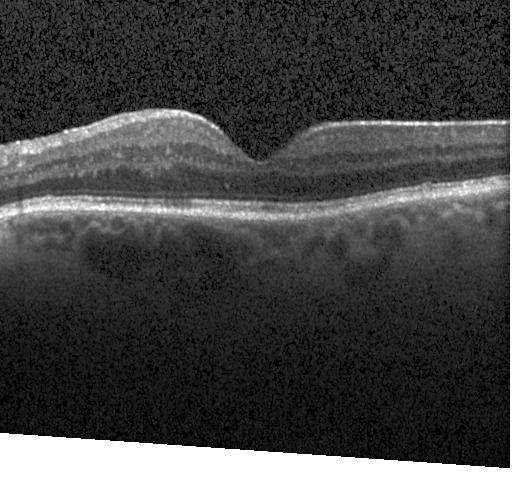 Horizontal scan through the fovea, optical coherence tomography scan, spectral-domain optical coherence tomography.
This B-scan demonstrates no choroidal neovascularization, no diabetic macular edema, and no drusen.